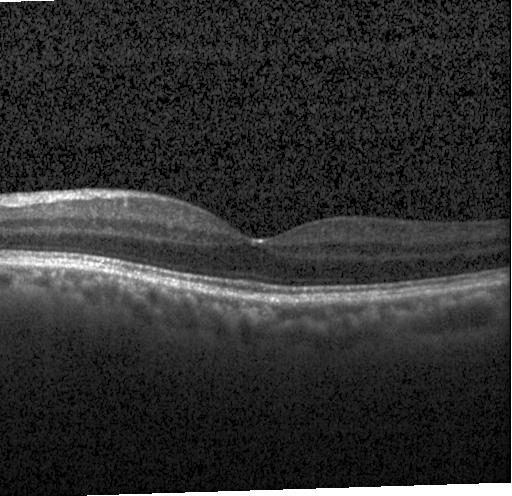

Macular OCT demonstrating no choroidal neovascularization, diabetic macular edema, or drusen.